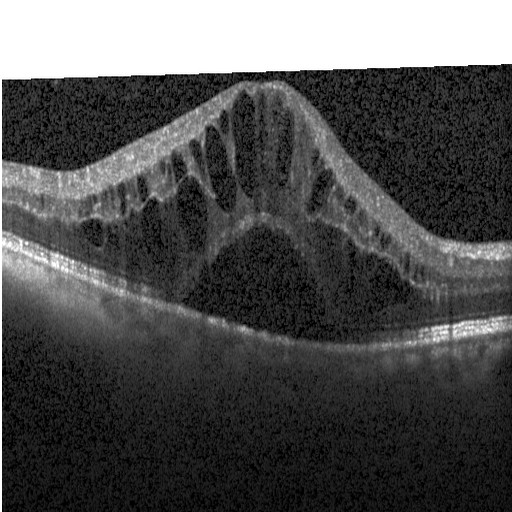
Spectral-domain OCT. Fovea-centered. Optical coherence tomography B-scan. Instrument: Heidelberg Spectralis. Impression: diabetic macular edema (DME).